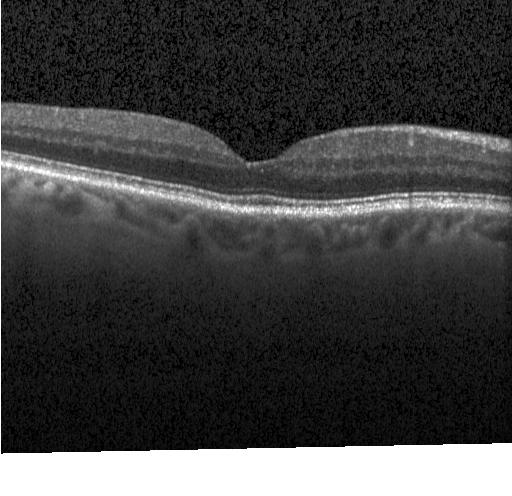

Heidelberg Spectralis OCT system; retinal OCT B-scan; horizontal scan through the fovea; spectral-domain OCT. No evidence of CNV, DME, or drusen.